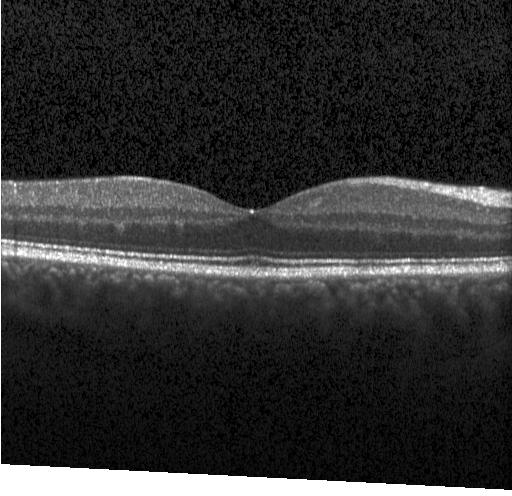 Finding: no choroidal neovascularization, diabetic macular edema, or drusen.